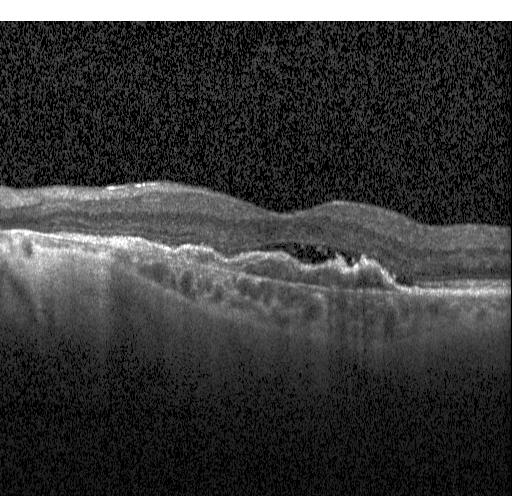
Retinal OCT cross-section showing a choroidal neovascular membrane.